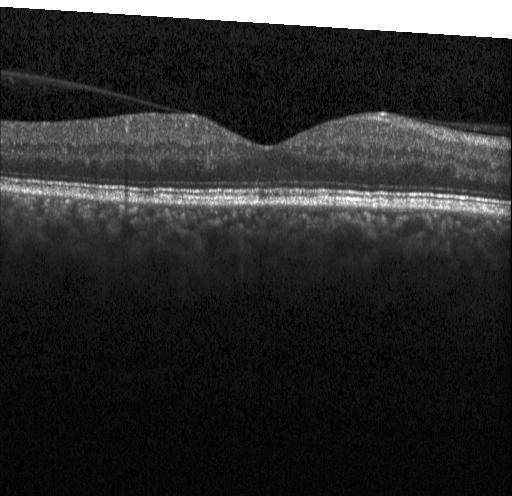

Optical coherence tomography B-scan.
Finding: no CNV, DME, or drusen.